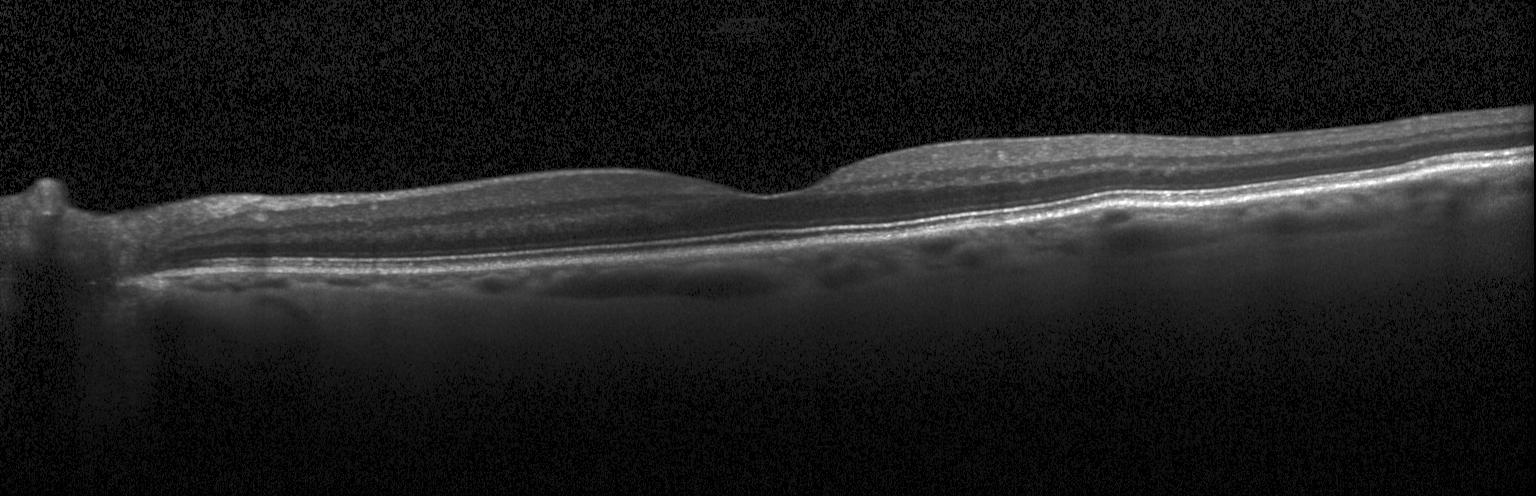 Optical coherence tomography B-scan. Diagnosis: no choroidal neovascularization, no diabetic macular edema, and no drusen.